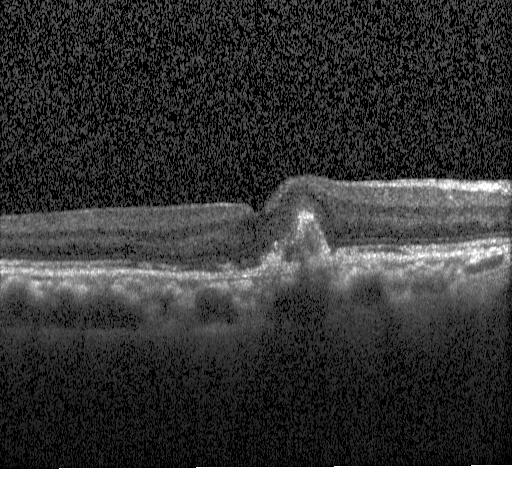
OCT line scan, Heidelberg Spectralis. Assessment: a choroidal neovascular membrane.